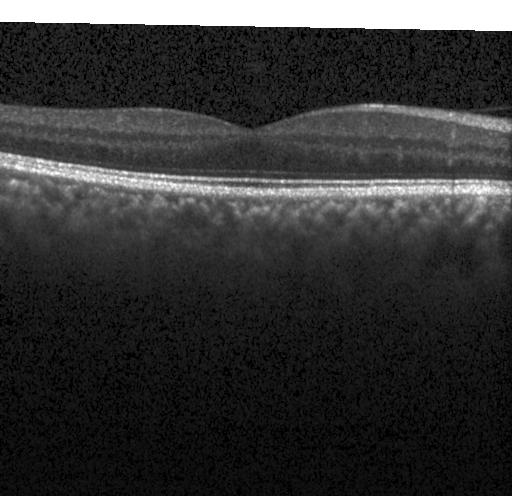
Heidelberg Spectralis OCT system · retinal OCT cross-section · through the macula · SD-OCT — Macular OCT: no evidence of choroidal neovascularization, diabetic macular edema, or drusen.